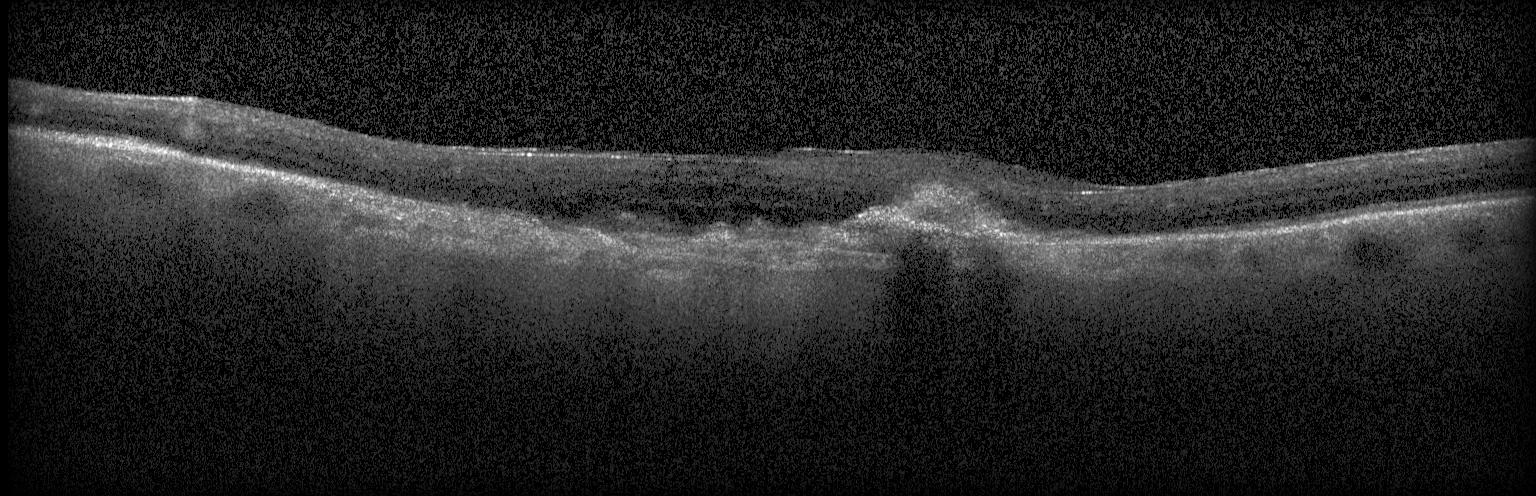

Dx: CNV.